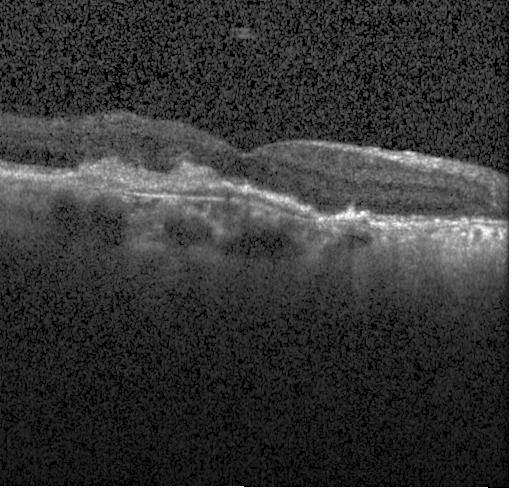

OCT line scan, Heidelberg Spectralis.
Impression: a choroidal neovascular membrane.